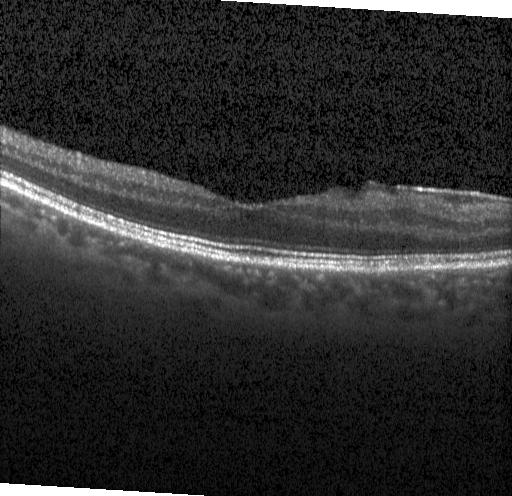 Spectral-domain OCT. Optical coherence tomography scan. Instrument: Heidelberg Spectralis. This B-scan demonstrates no evidence of choroidal neovascularization, diabetic macular edema, or drusen.